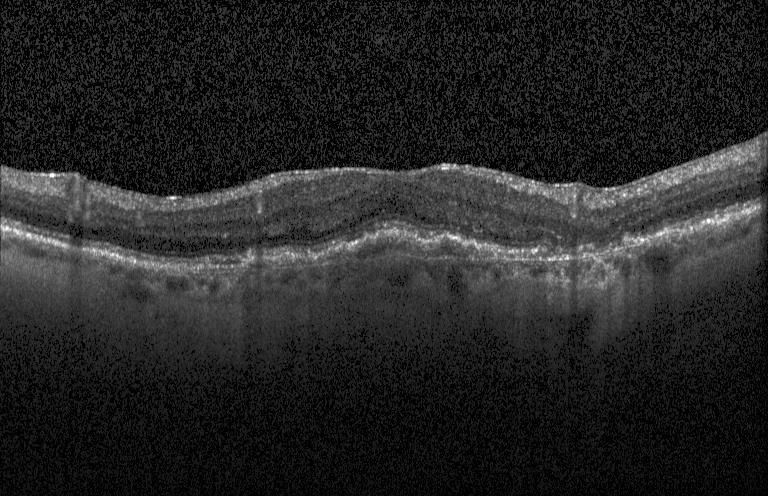
OCT B-scan. Spectral-domain OCT. Fovea-centered.
Impression: CNV.